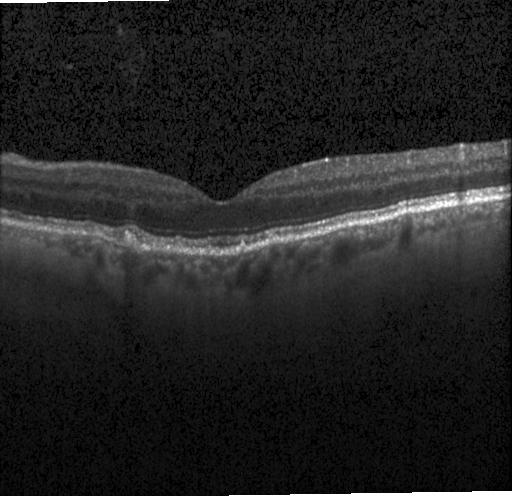 SD-OCT. Optical coherence tomography scan
This B-scan demonstrates multiple drusen.